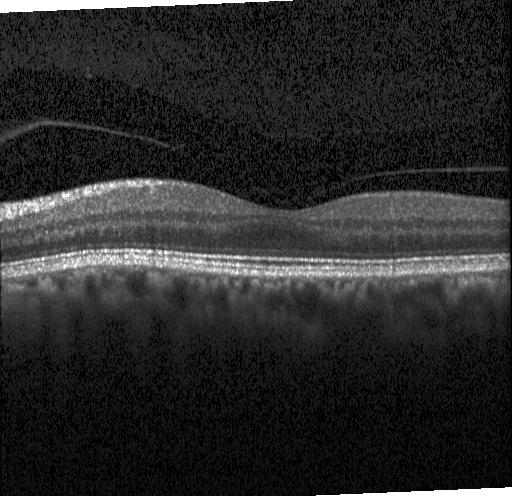 Fovea-centered, spectral-domain OCT, OCT B-scan, acquired on a Heidelberg Spectralis
Finding: no choroidal neovascularization, no diabetic macular edema, and no drusen.